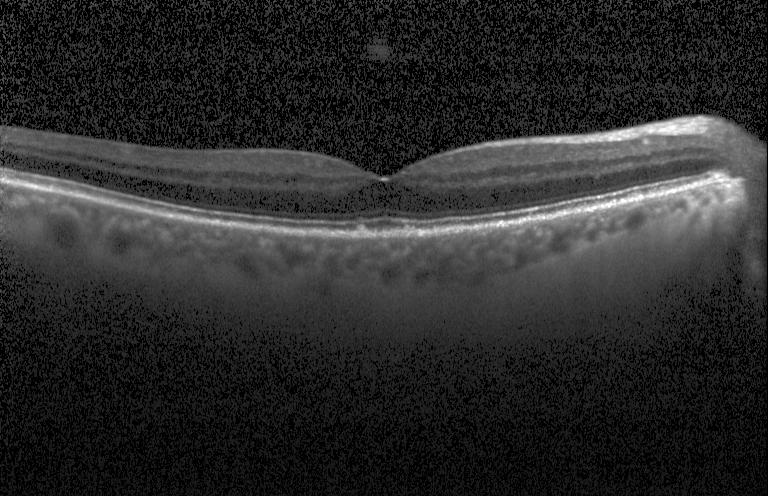

Diagnosis: drusen.